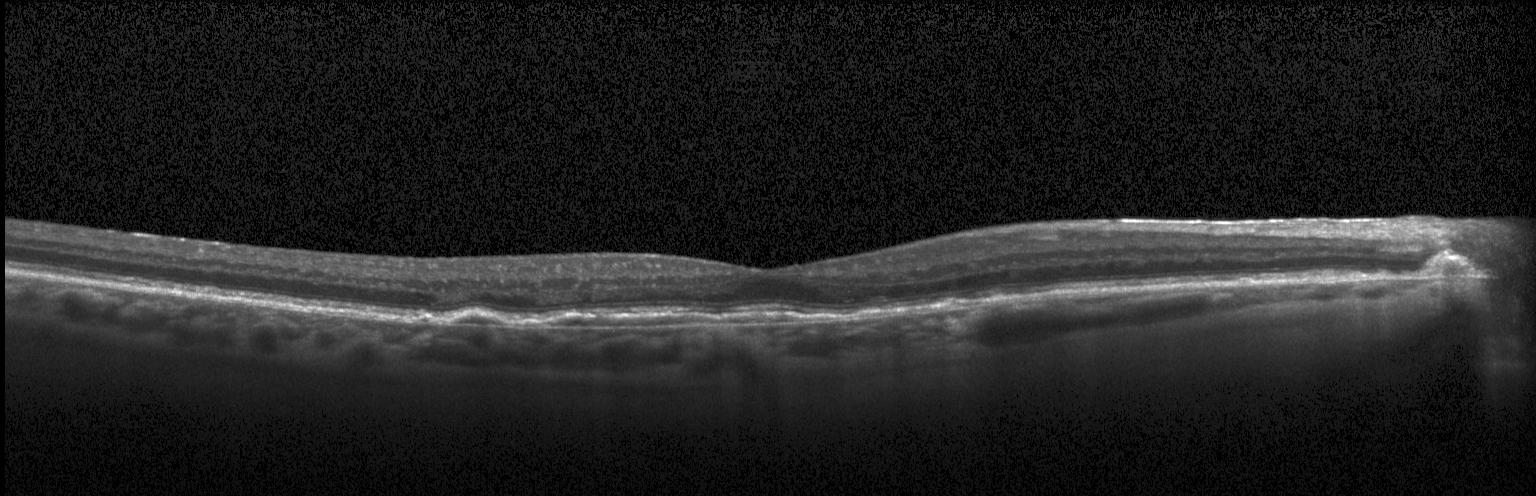

Retinal OCT B-scan.
Choroidal neovascularization (CNV).